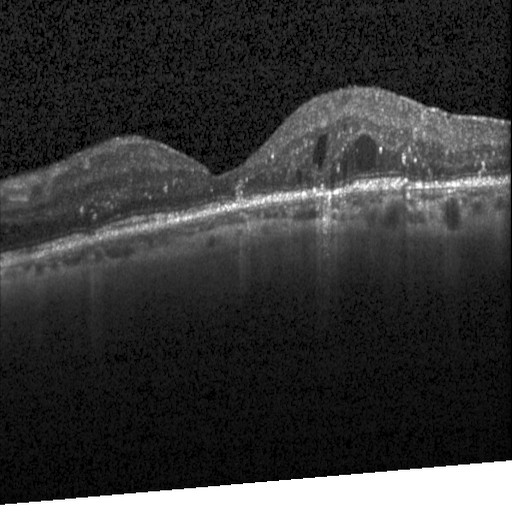

Assessment: diabetic macular edema.